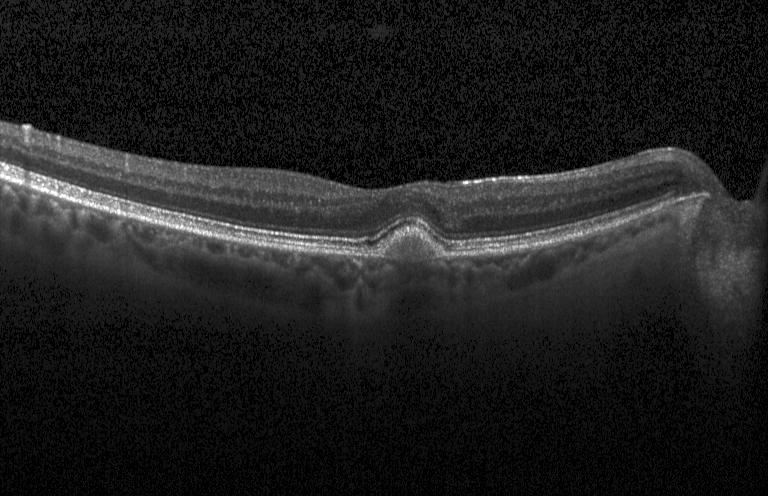

Optical coherence tomography scan. Fovea-centered. Acquired on a Heidelberg Spectralis.
Diagnosis: drusen.